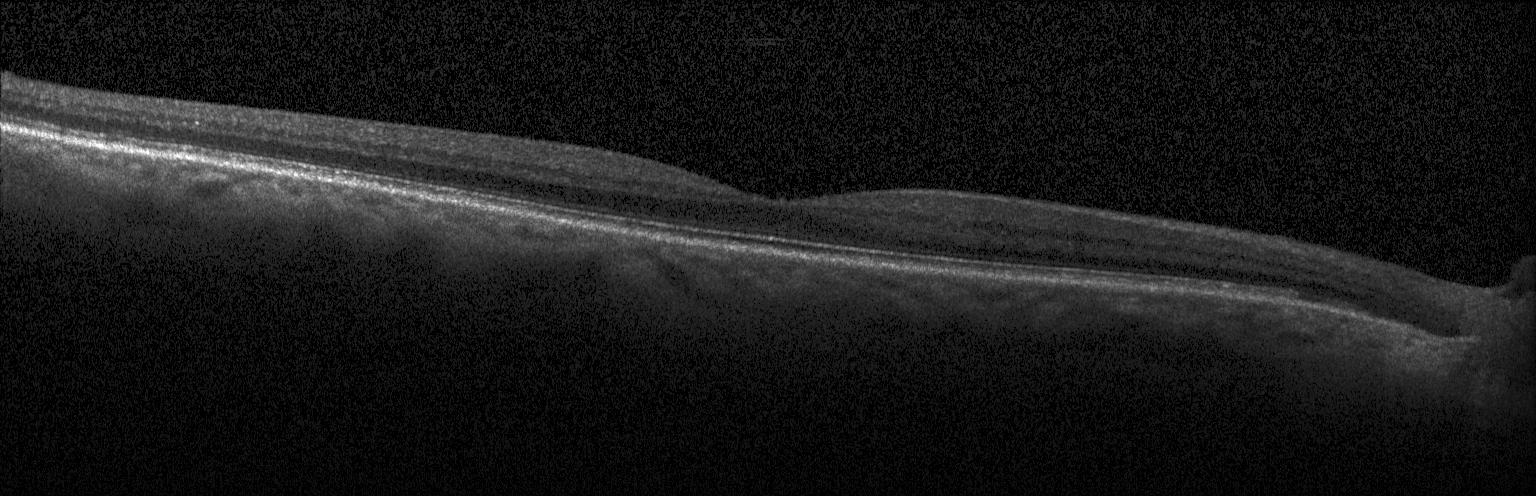

Heidelberg Spectralis OCT system · fovea-centered · spectral-domain optical coherence tomography · retinal OCT cross-section
The scan shows no evidence of choroidal neovascularization, diabetic macular edema, or drusen.